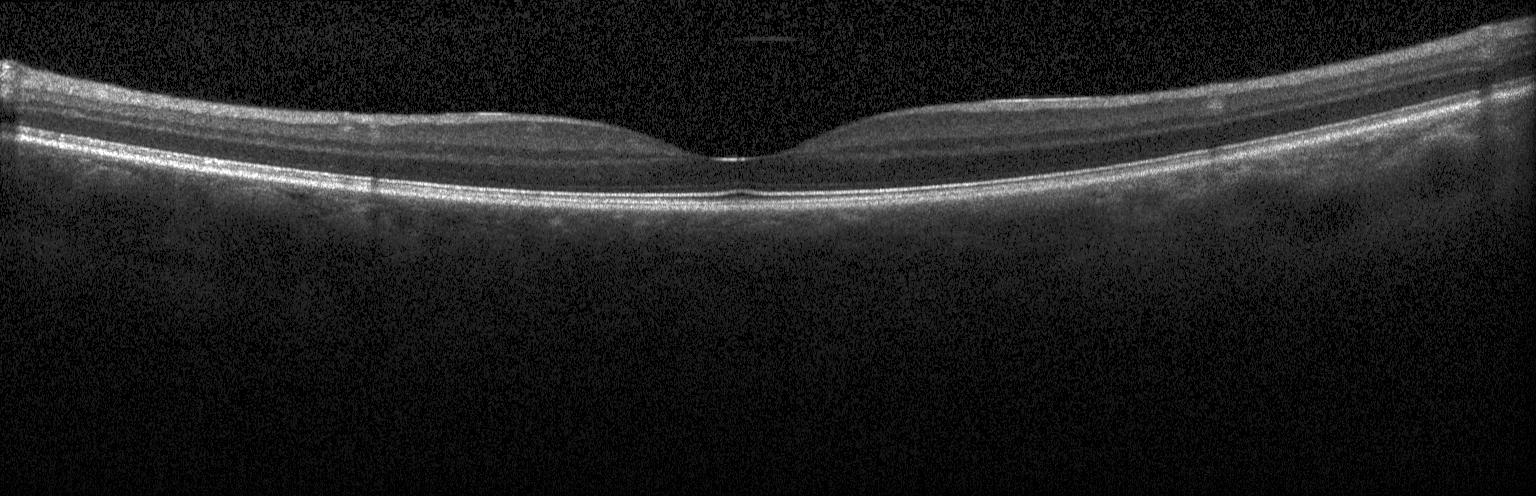
Macular scan · OCT line scan · spectral-domain OCT. Diagnosis: no evidence of choroidal neovascularization, diabetic macular edema, or drusen.